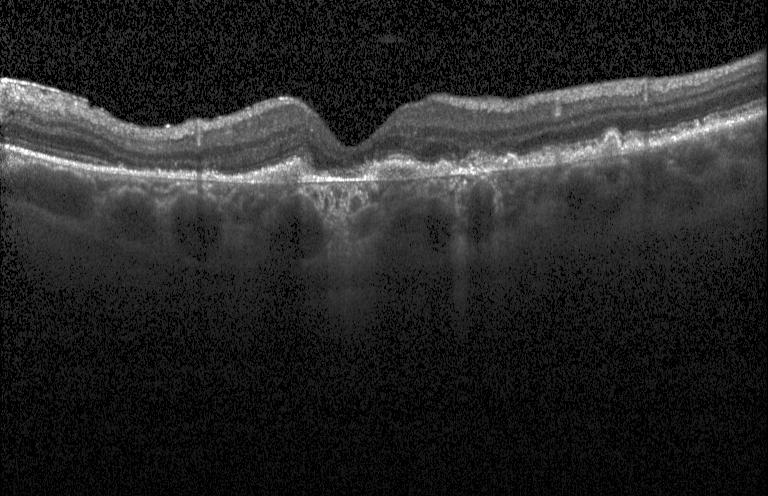
Retinal OCT B-scan
Finding: CNV.